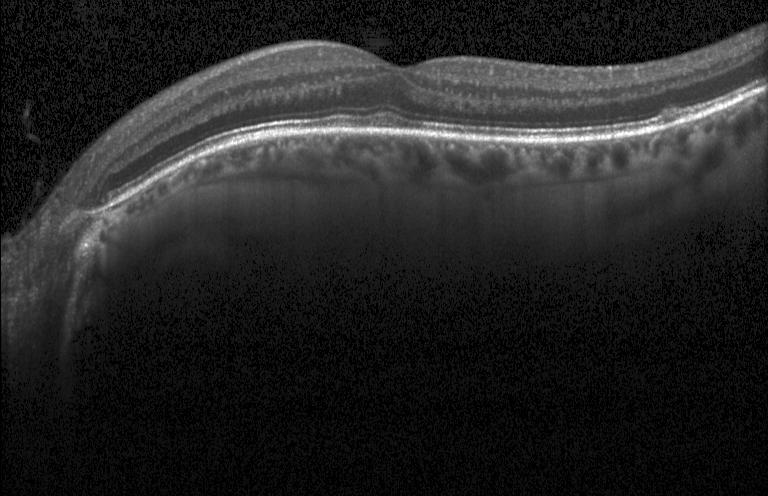

Retinal OCT cross-section; spectral-domain OCT; Heidelberg Spectralis OCT system.
No choroidal neovascularization, diabetic macular edema, or drusen.